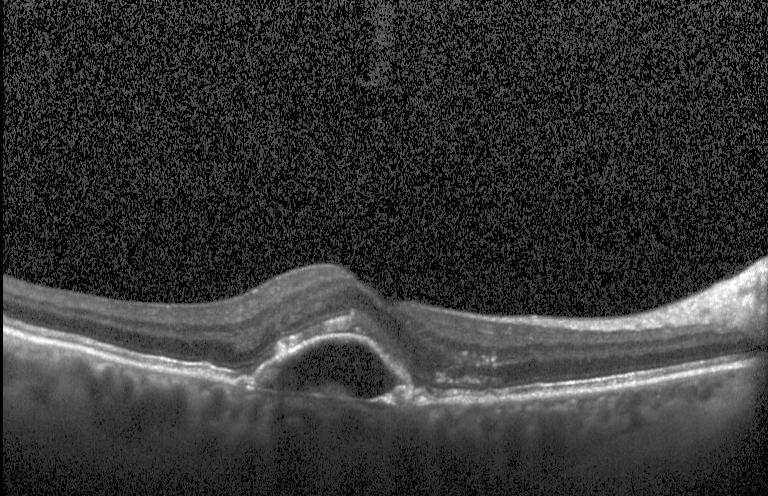
Finding: a choroidal neovascular membrane.